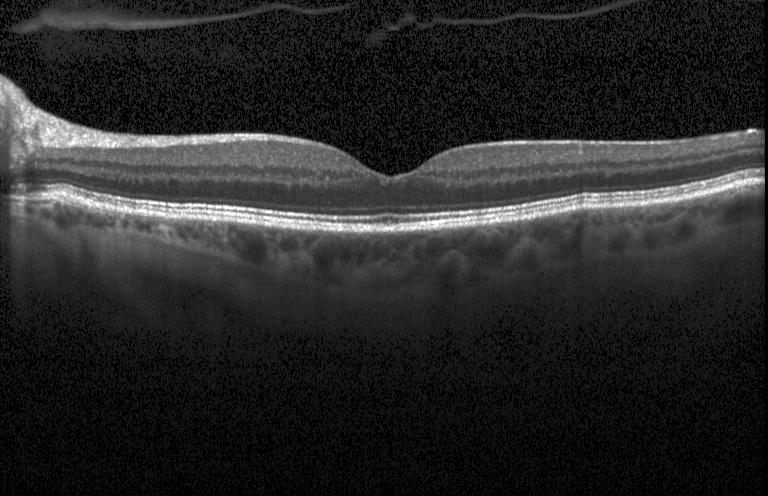 Spectral-domain OCT, OCT B-scan, instrument: Heidelberg Spectralis. Diagnosis: no CNV, no DME, and no drusen.